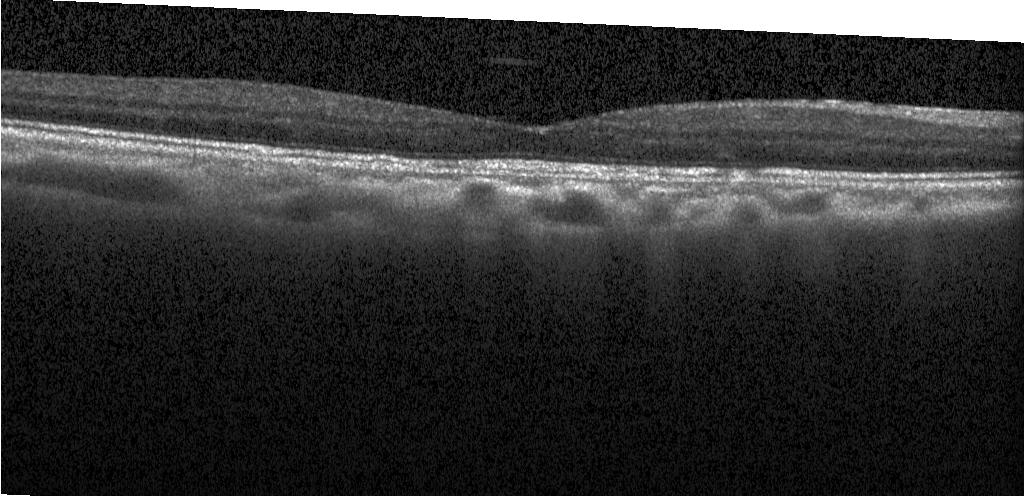

Retinal OCT cross-section showing neither CNV, DME, nor drusen.